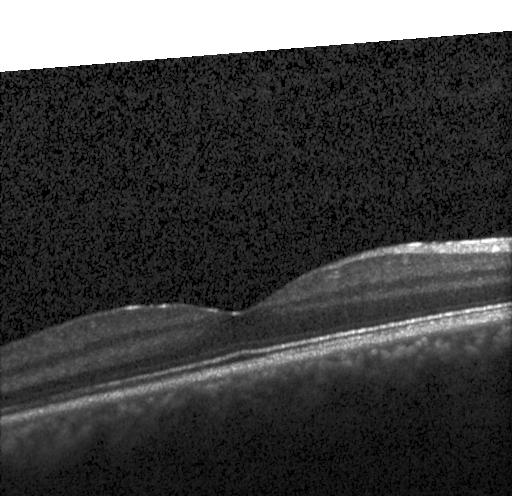

Instrument: Heidelberg Spectralis. OCT B-scan
OCT finding: no CNV, no DME, and no drusen.